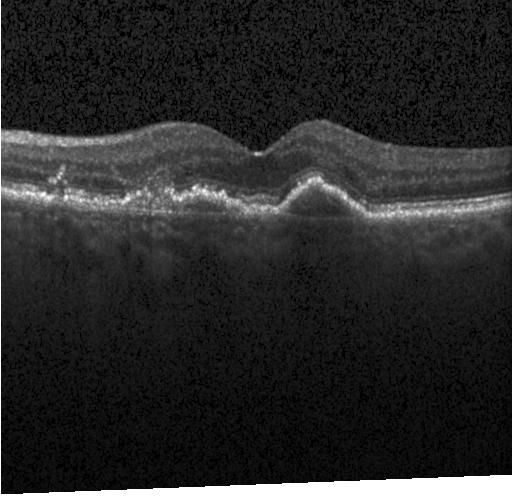
Macular scan; instrument: Heidelberg Spectralis; spectral-domain optical coherence tomography; OCT B-scan. Choroidal neovascularization.